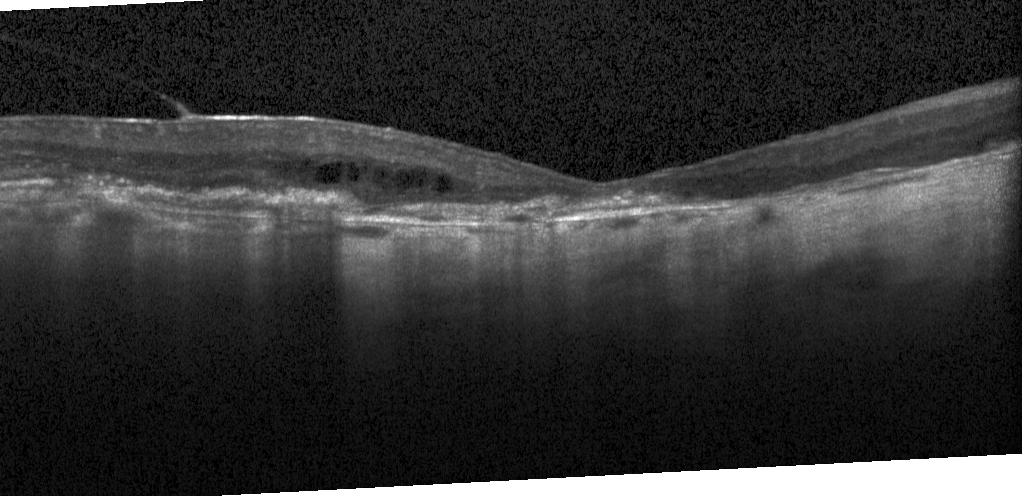
Dx: choroidal neovascularization (CNV).